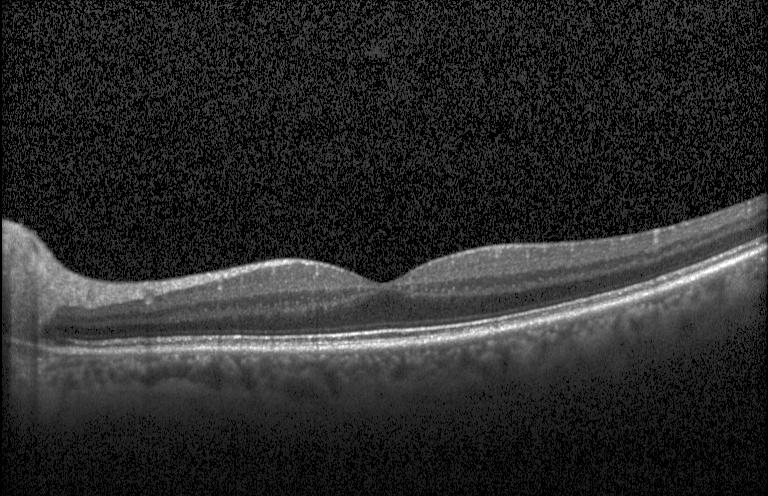

Spectral-domain OCT, centered on the fovea, instrument: Heidelberg Spectralis, retinal OCT cross-section. OCT finding: no choroidal neovascularization, no diabetic macular edema, and no drusen.